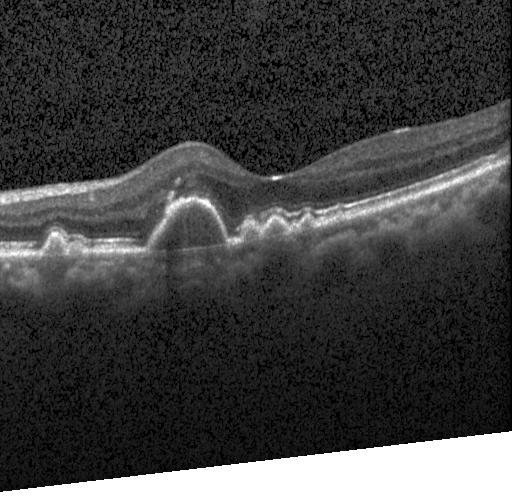
Instrument: Heidelberg Spectralis. Fovea-centered. Spectral-domain optical coherence tomography. OCT line scan. Impression: sub-RPE drusenoid deposits.